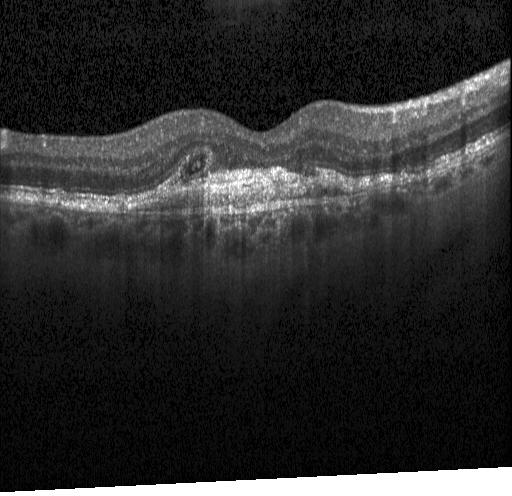

Instrument: Heidelberg Spectralis, OCT line scan, fovea-centered.
Finding: a choroidal neovascular membrane.